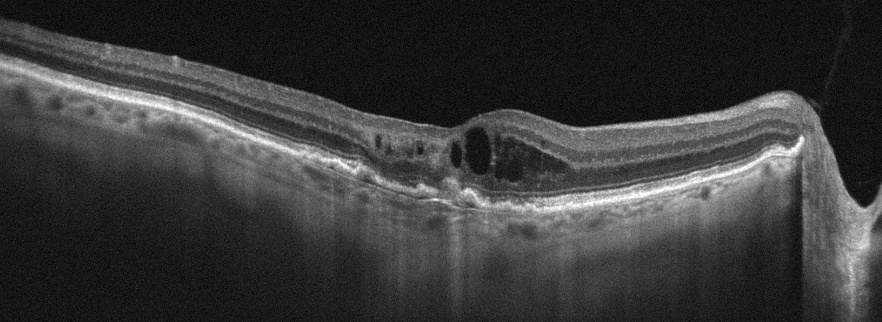
Fovea-centered, retinal OCT B-scan, acquired on an Optovue Avanti RTVue XR, right eye.
Diagnosis: age-related macular degeneration (AMD).